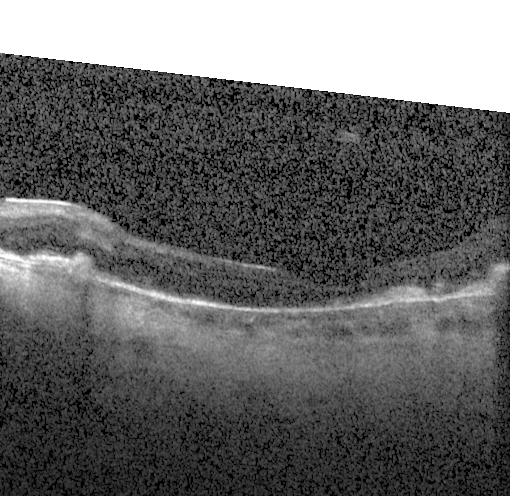
Spectral-domain OCT. OCT line scan. Heidelberg Spectralis. Fovea-centered
Macular OCT: choroidal neovascularization (CNV).